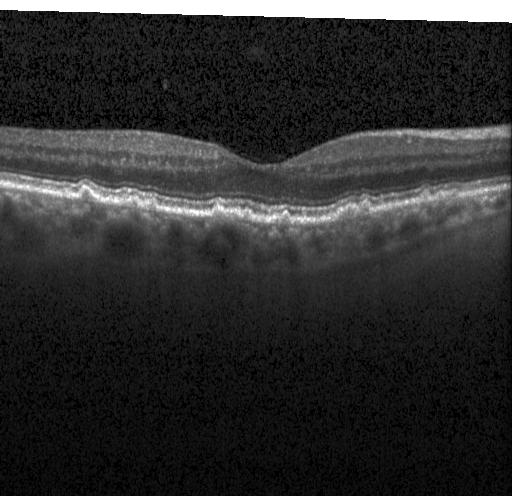 Diagnosis: multiple drusen.